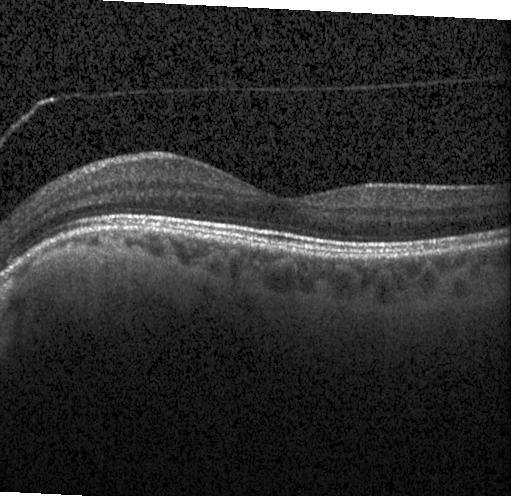 No choroidal neovascularization, diabetic macular edema, or drusen.